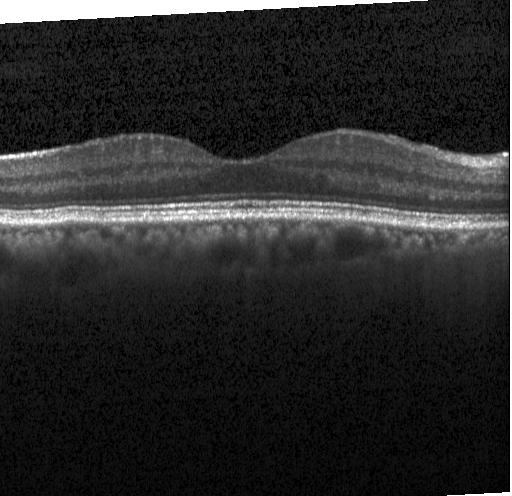

Horizontal scan through the fovea · spectral-domain OCT · OCT B-scan — Dx: no CNV, DME, or drusen.